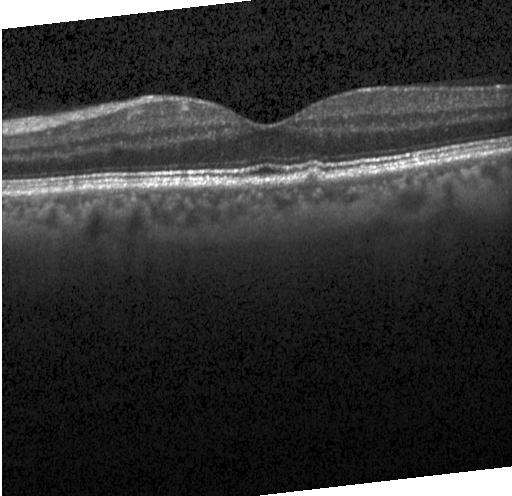
Retinal OCT cross-section. Macular OCT: sub-RPE drusenoid deposits.